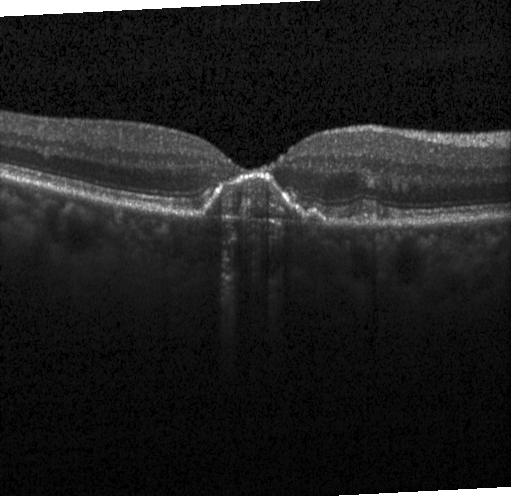
Horizontal scan through the fovea, spectral-domain optical coherence tomography, optical coherence tomography B-scan.
Dx: a choroidal neovascular membrane.